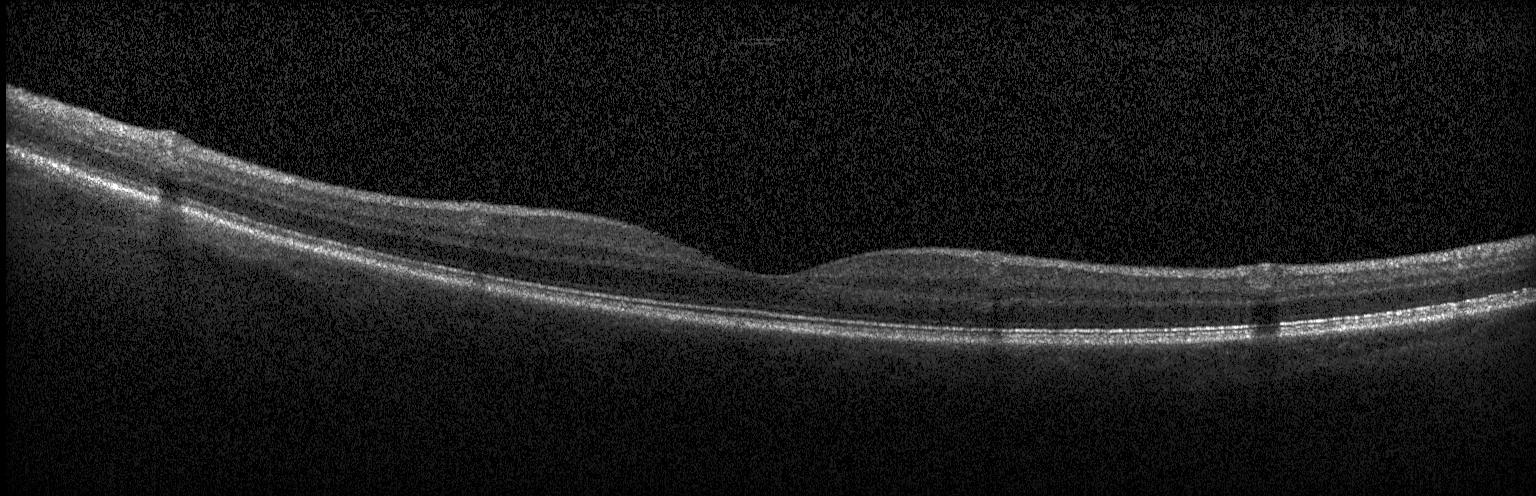

Instrument: Heidelberg Spectralis, spectral-domain optical coherence tomography, retinal OCT cross-section. Macular OCT: no choroidal neovascularization, no diabetic macular edema, and no drusen.